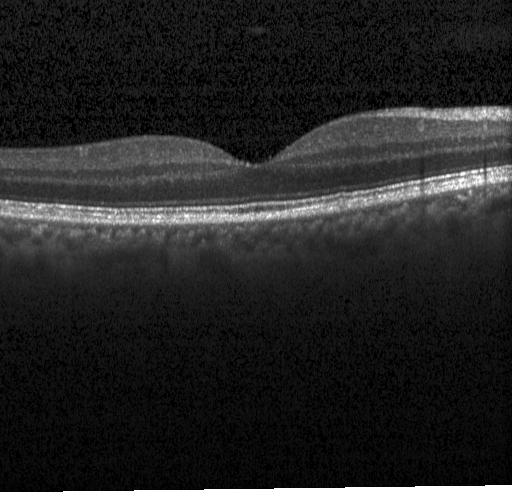
OCT finding: neither CNV, DME, nor drusen.